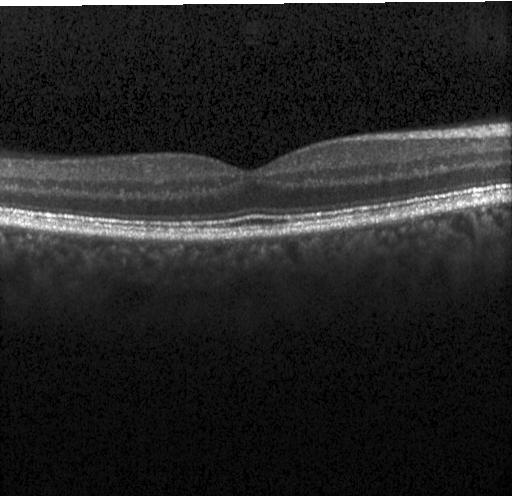
Retinal OCT cross-section showing no choroidal neovascularization, no diabetic macular edema, and no drusen.